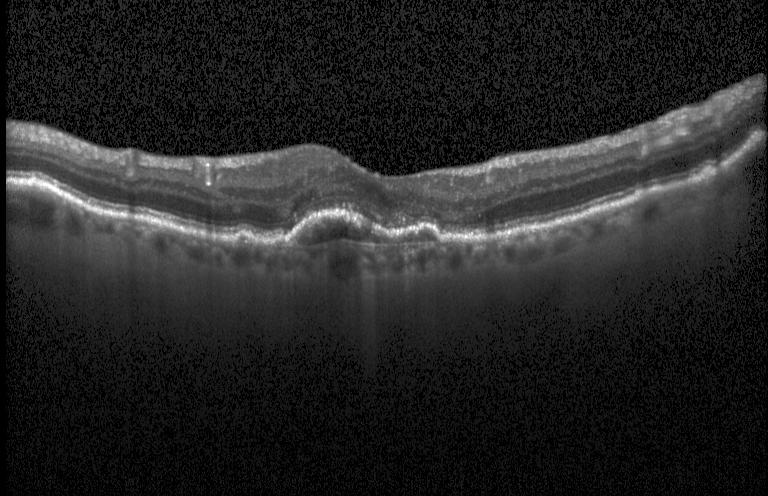 Spectral-domain optical coherence tomography. Instrument: Heidelberg Spectralis. Optical coherence tomography B-scan.
Impression: a choroidal neovascular membrane.